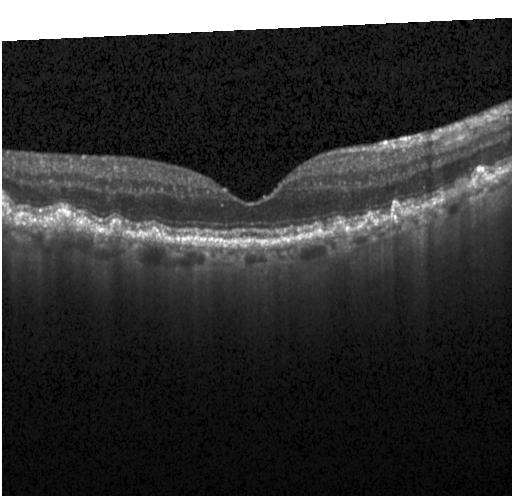 Macular OCT: multiple drusen.